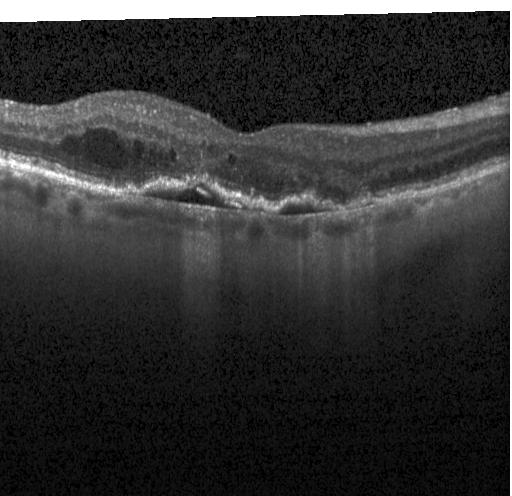 Fovea-centered. Heidelberg Spectralis OCT system. Optical coherence tomography B-scan
Dx: a choroidal neovascular membrane.